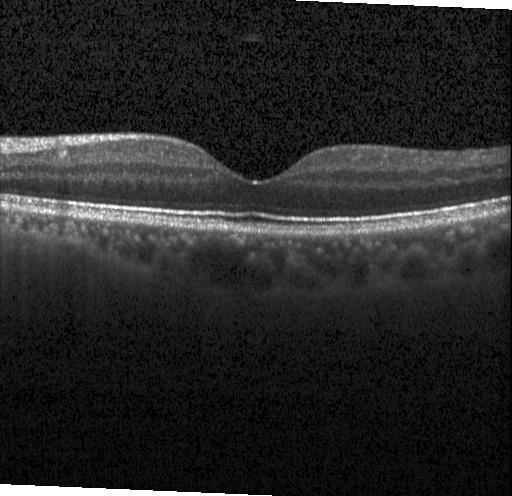
Optical coherence tomography B-scan, instrument: Heidelberg Spectralis. Diagnosis: no CNV, DME, or drusen.